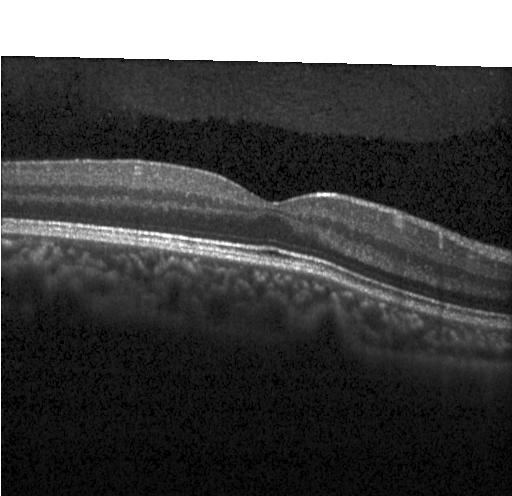

OCT B-scan showing no CNV, DME, or drusen.